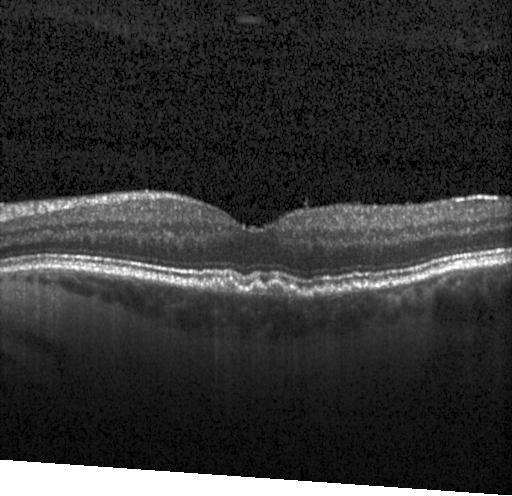
OCT B-scan showing multiple drusen.